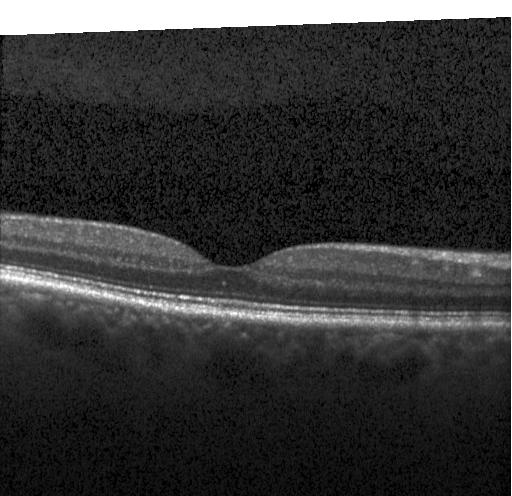
SD-OCT. Horizontal scan through the fovea. Optical coherence tomography scan
Finding: neither choroidal neovascularization, diabetic macular edema, nor drusen.